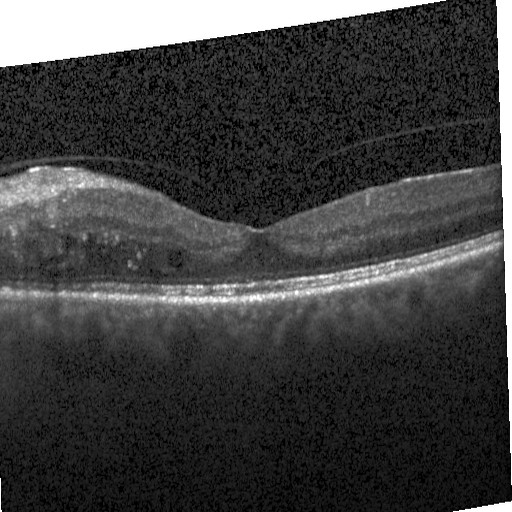

Retinal OCT B-scan — Diabetic macular edema (DME).